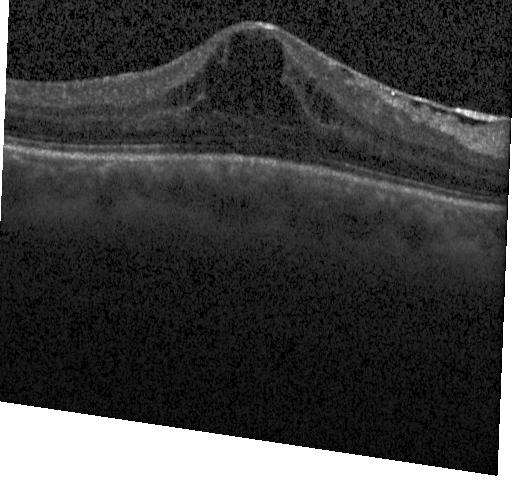

Retinal OCT cross-section. Fovea-centered. Heidelberg Spectralis OCT system.
DME.